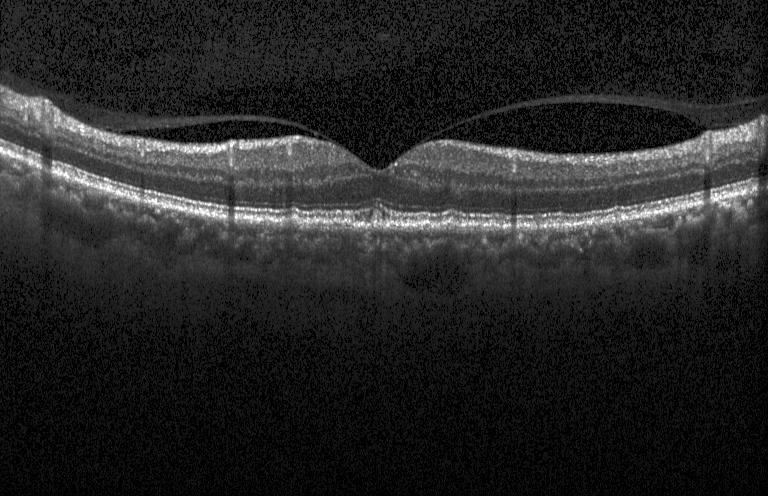 Acquired on a Heidelberg Spectralis, optical coherence tomography scan, through the macula. Dx: sub-RPE drusenoid deposits.